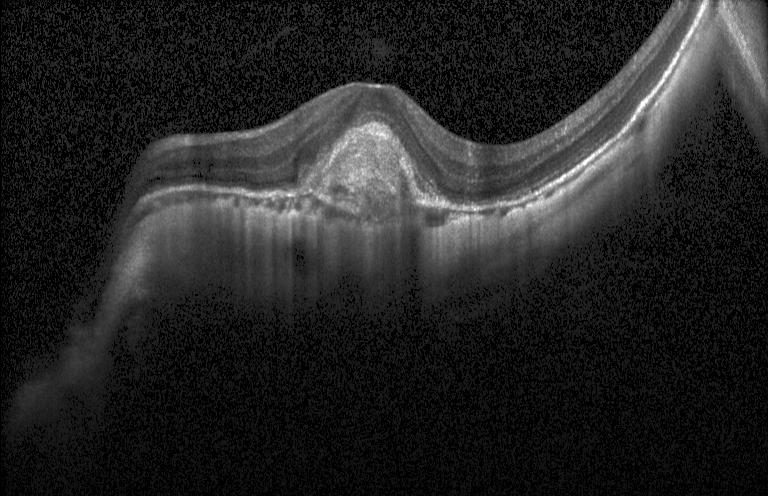
Optical coherence tomography scan
This B-scan demonstrates a choroidal neovascular membrane.